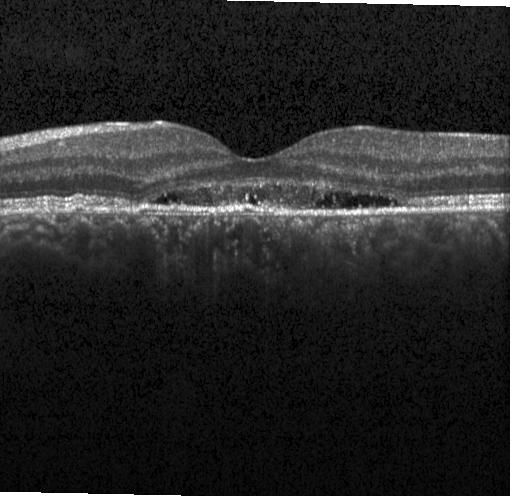 OCT line scan. Fovea-centered. SD-OCT — This B-scan demonstrates a choroidal neovascular membrane.